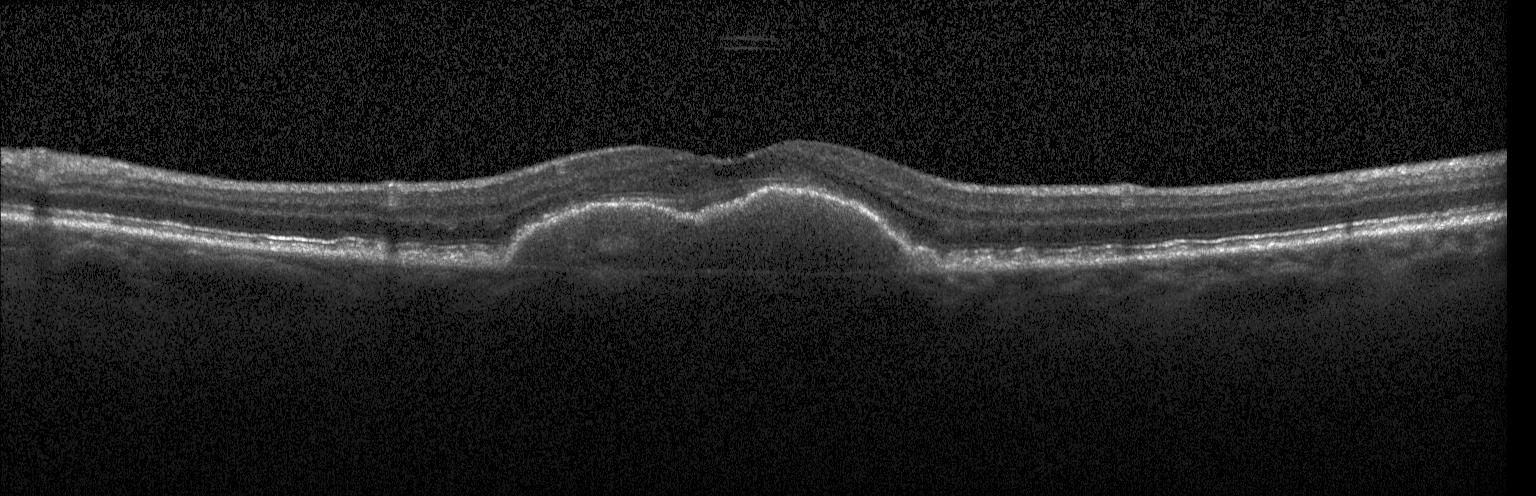

The scan shows choroidal neovascularization (CNV).